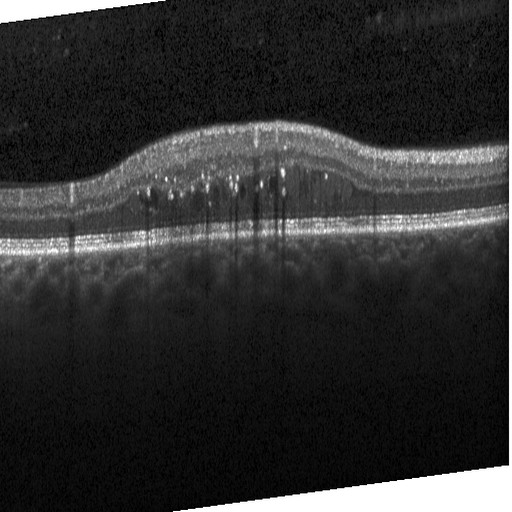
OCT B-scan showing diabetic macular edema.